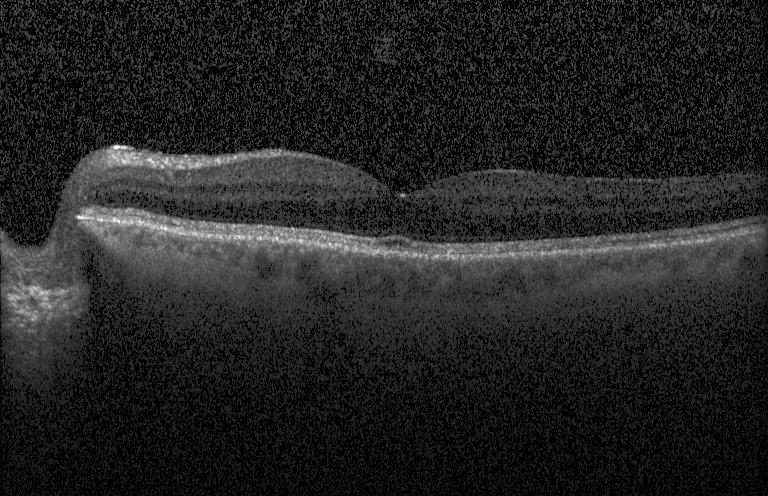 Dx: no choroidal neovascularization, no diabetic macular edema, and no drusen.